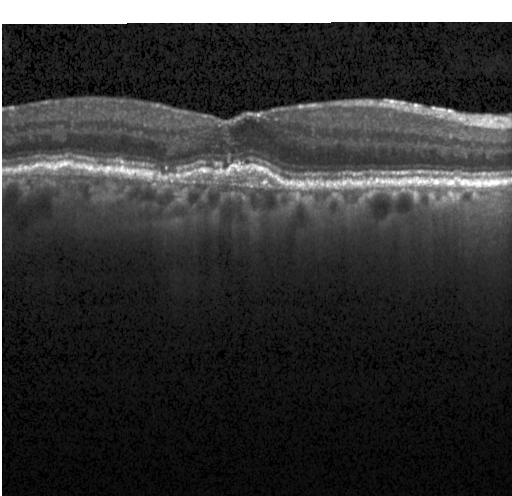 Retinal OCT cross-section — OCT finding: choroidal neovascularization (CNV).